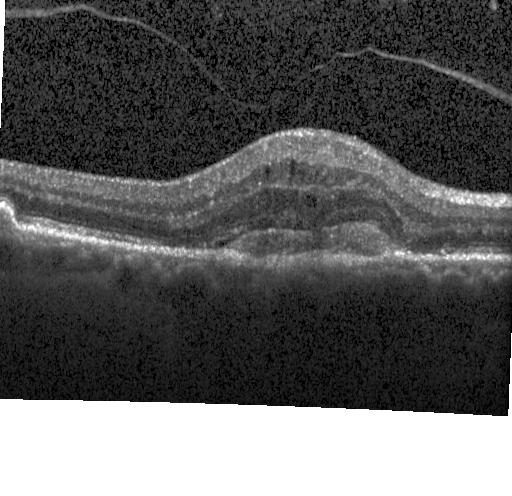
SD-OCT; OCT B-scan — Macular OCT: a choroidal neovascular membrane.